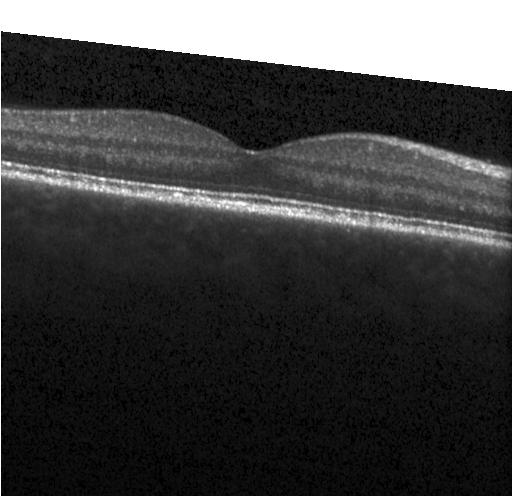
OCT line scan, instrument: Heidelberg Spectralis — No choroidal neovascularization, no diabetic macular edema, and no drusen.